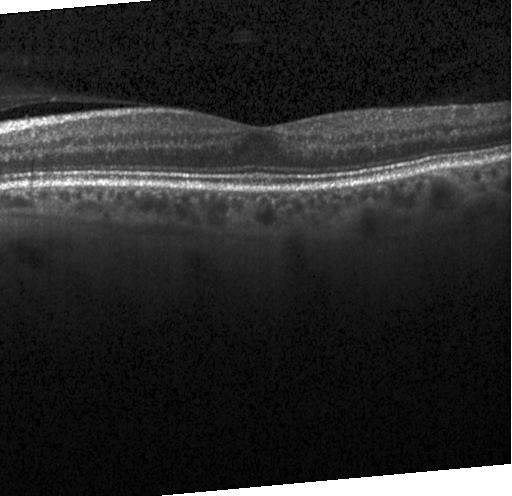 The scan shows neither CNV, DME, nor drusen.